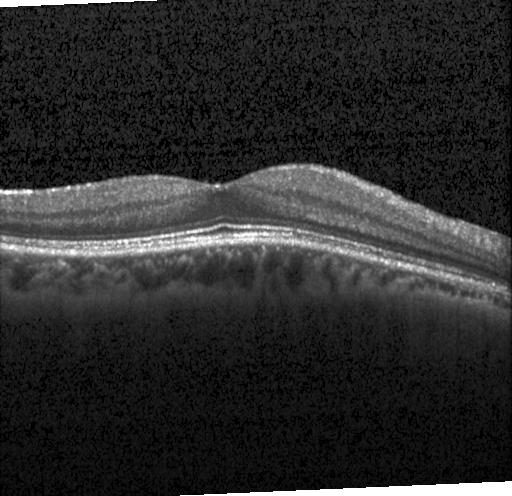

Dx: no evidence of CNV, DME, or drusen.